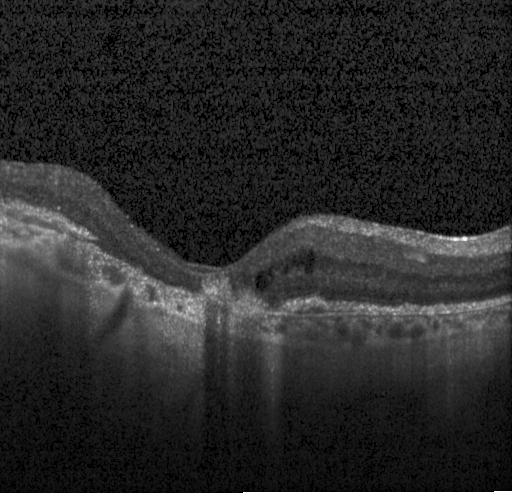 OCT scan showing a choroidal neovascular membrane.